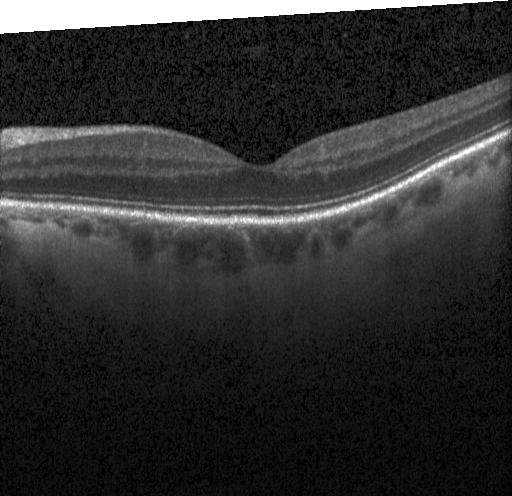 The scan shows neither choroidal neovascularization, diabetic macular edema, nor drusen.